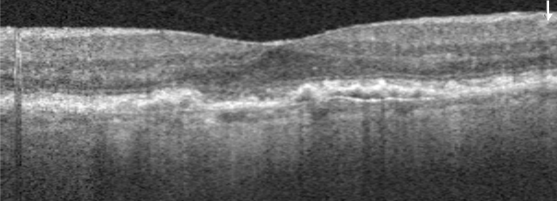 Fovea-centered, optical coherence tomography scan. The scan shows age-related macular degeneration.